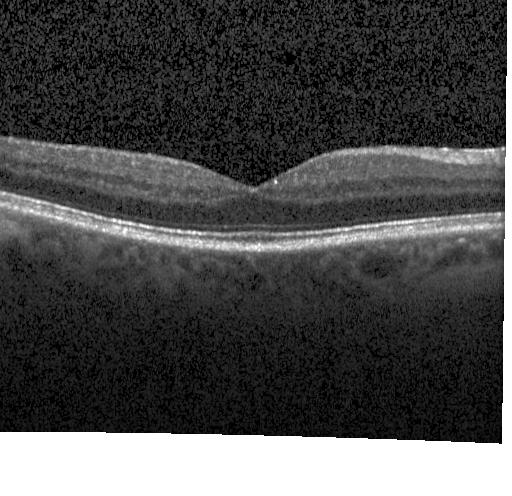 Retinal OCT cross-section showing neither CNV, DME, nor drusen.